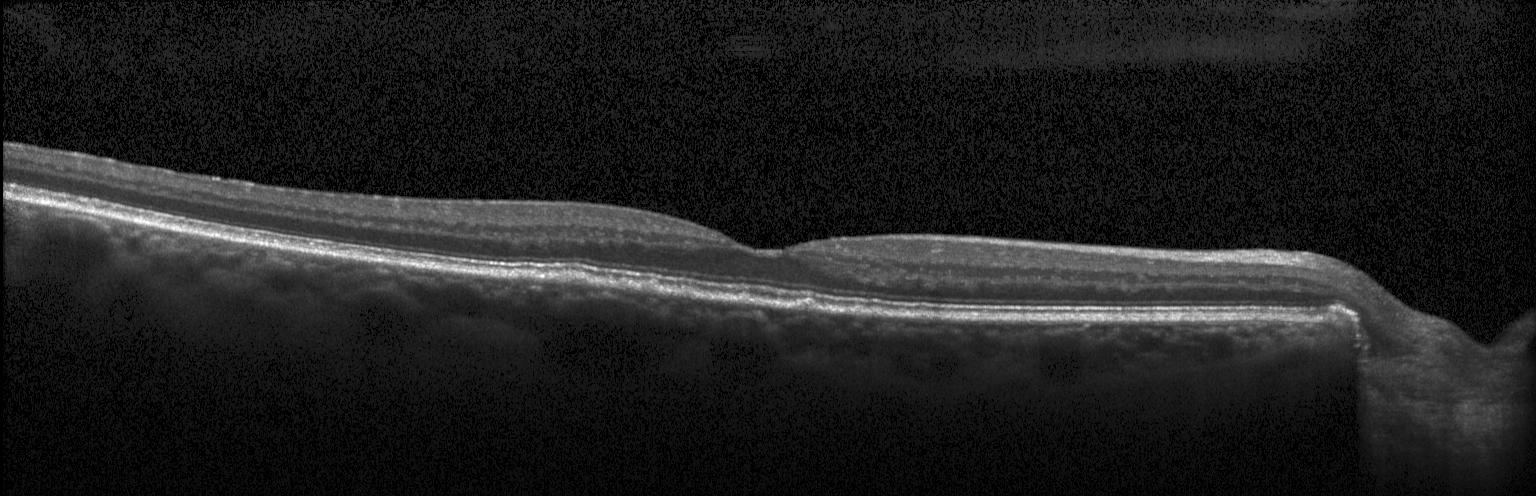

SD-OCT. Optical coherence tomography scan. Drusen.